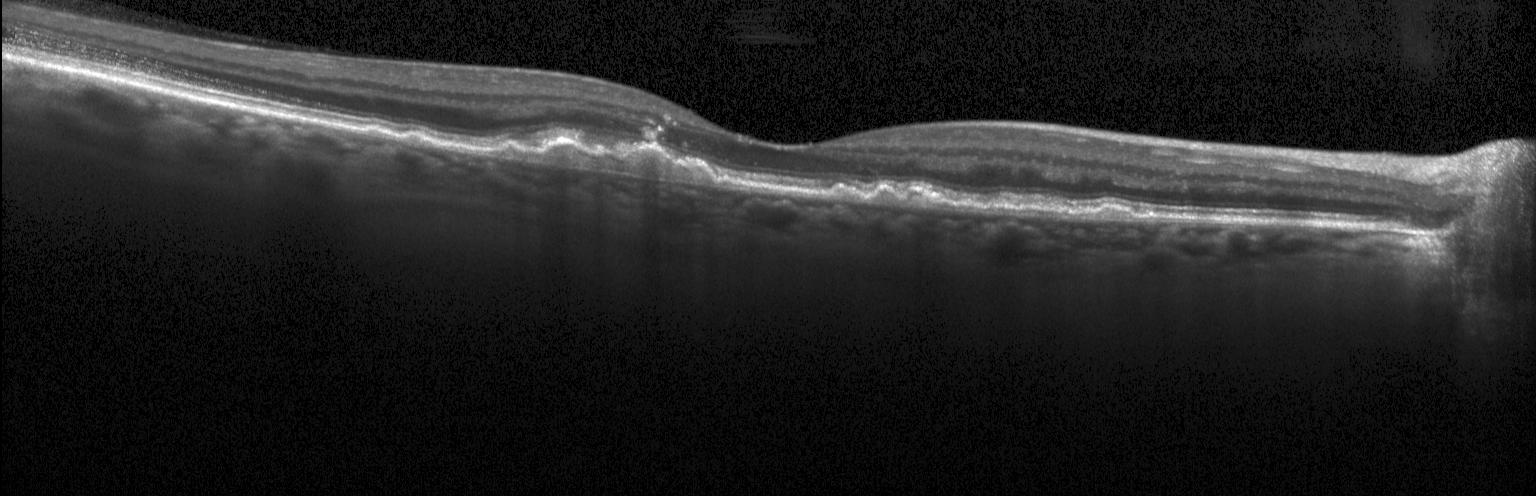 Optical coherence tomography B-scan · spectral-domain OCT · acquired on a Heidelberg Spectralis — Diagnosis: choroidal neovascularization.